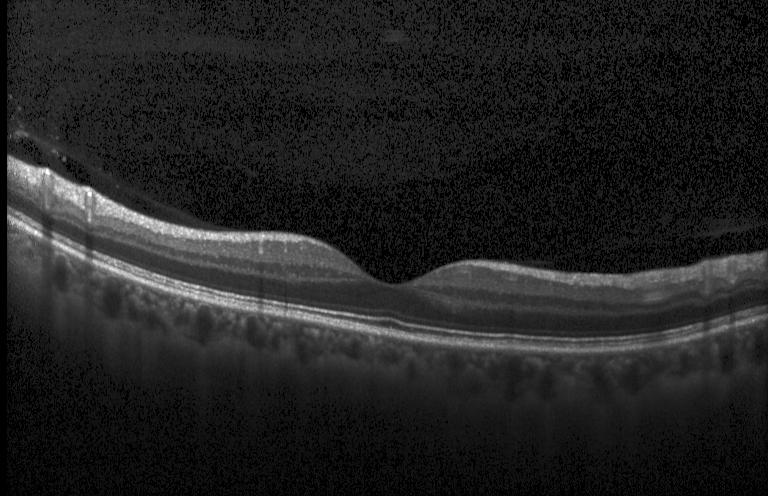

OCT finding: no evidence of choroidal neovascularization, diabetic macular edema, or drusen.